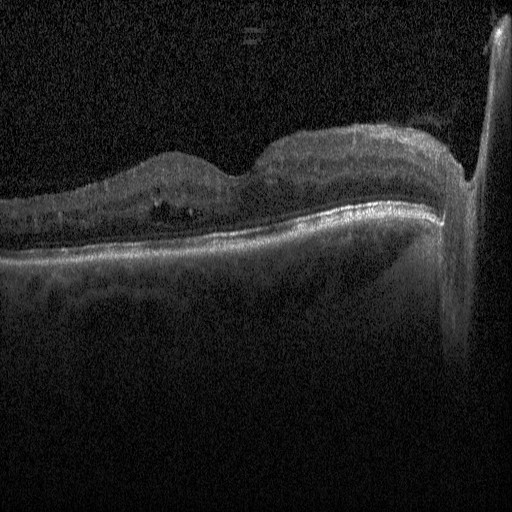 Diabetic macular edema (DME).